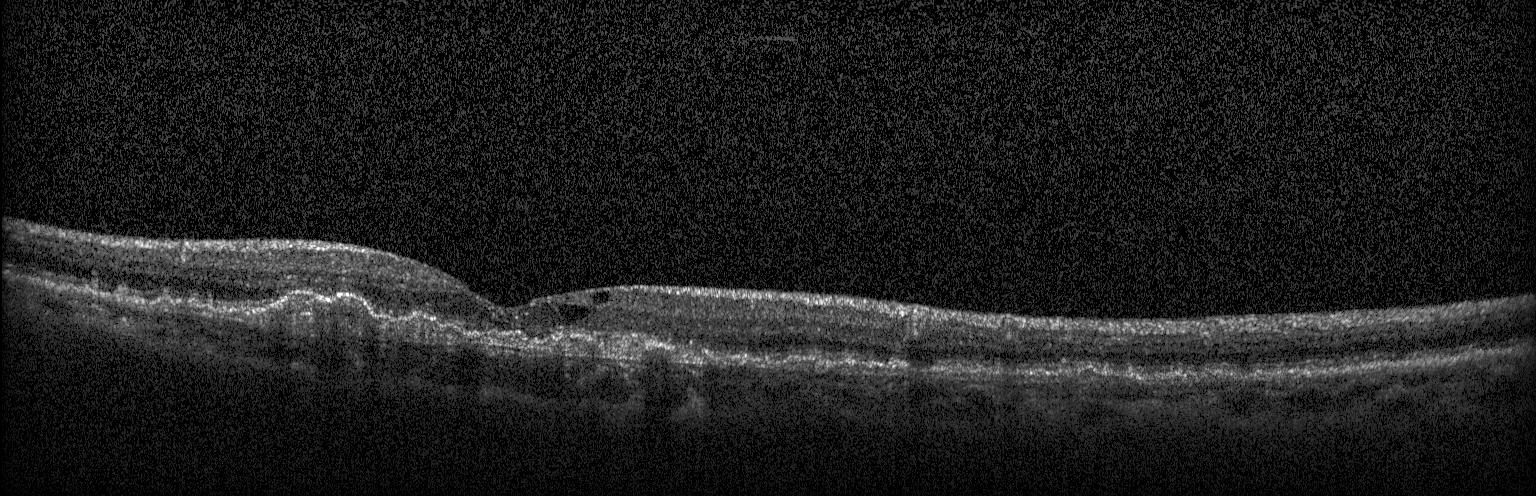

Fovea-centered, instrument: Heidelberg Spectralis, OCT line scan, SD-OCT
Diagnosis: choroidal neovascularization (CNV).